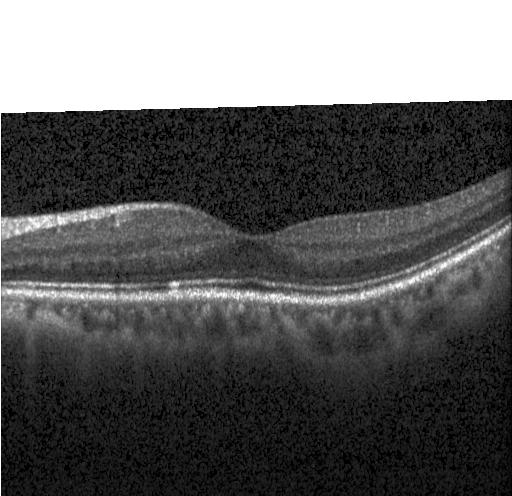

SD-OCT · instrument: Heidelberg Spectralis · macular scan · retinal OCT B-scan — Finding: no choroidal neovascularization, no diabetic macular edema, and no drusen.